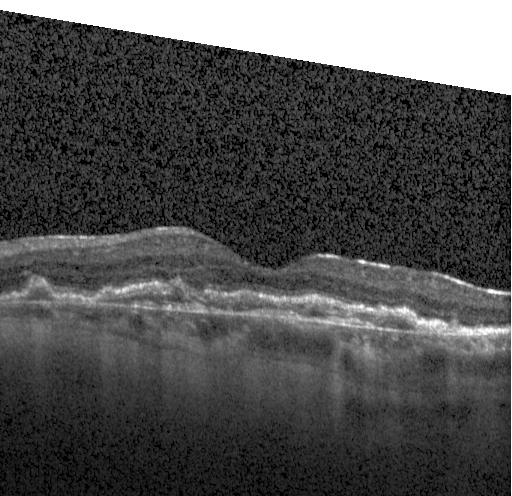 Spectral-domain optical coherence tomography, horizontal scan through the fovea, Heidelberg Spectralis OCT system, OCT B-scan.
Macular OCT: a choroidal neovascular membrane.